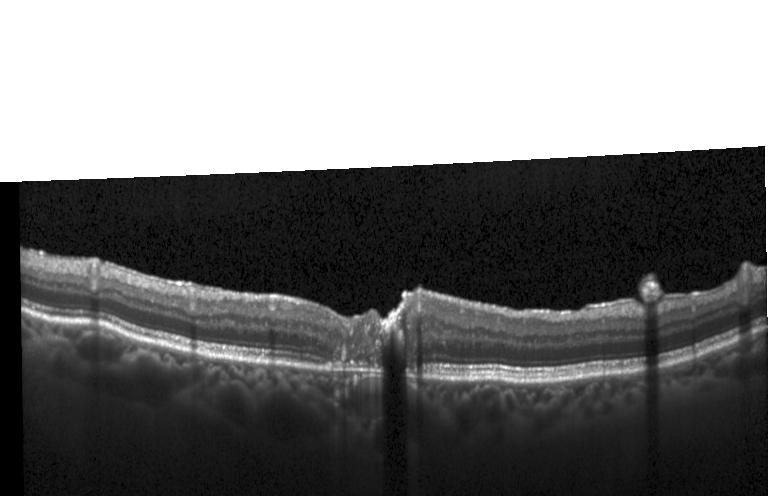 Finding: CNV.